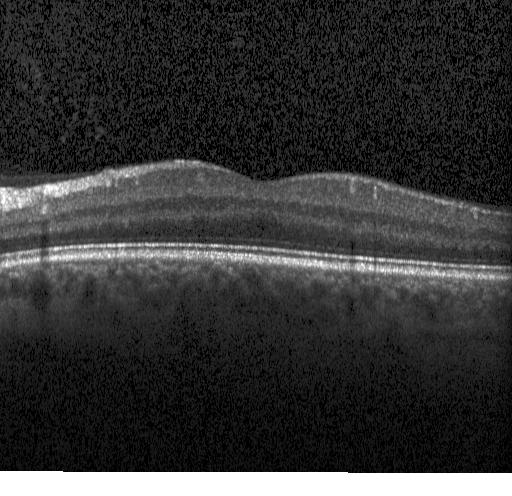 Acquired on a Heidelberg Spectralis; OCT line scan; centered on the fovea; spectral-domain optical coherence tomography. The scan shows no CNV, DME, or drusen.